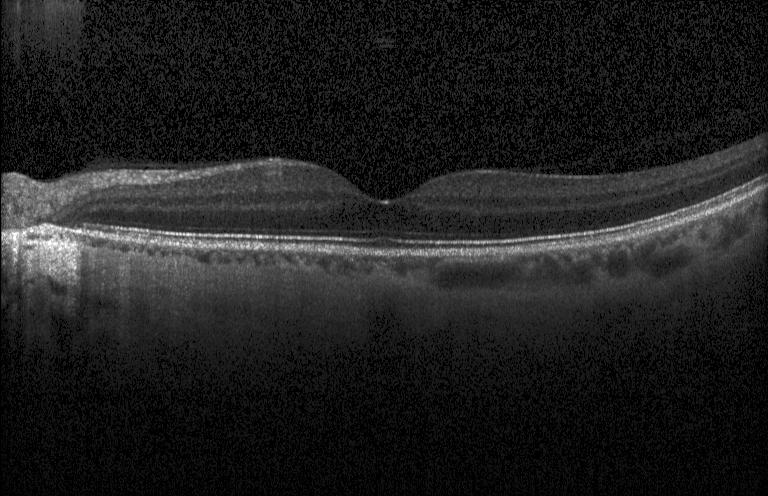 Heidelberg Spectralis, OCT B-scan, spectral-domain OCT, horizontal scan through the fovea — Assessment: no choroidal neovascularization, diabetic macular edema, or drusen.